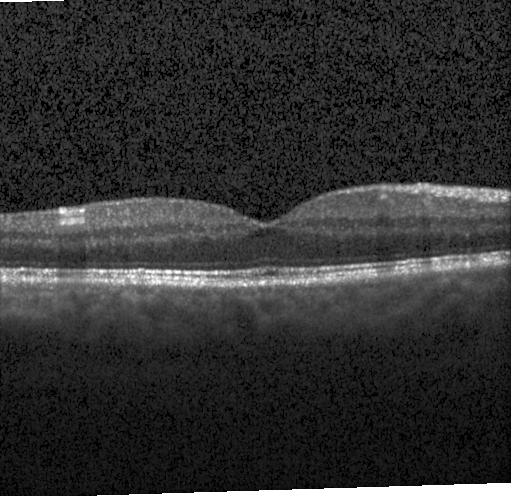

Optical coherence tomography scan. No choroidal neovascularization, diabetic macular edema, or drusen.